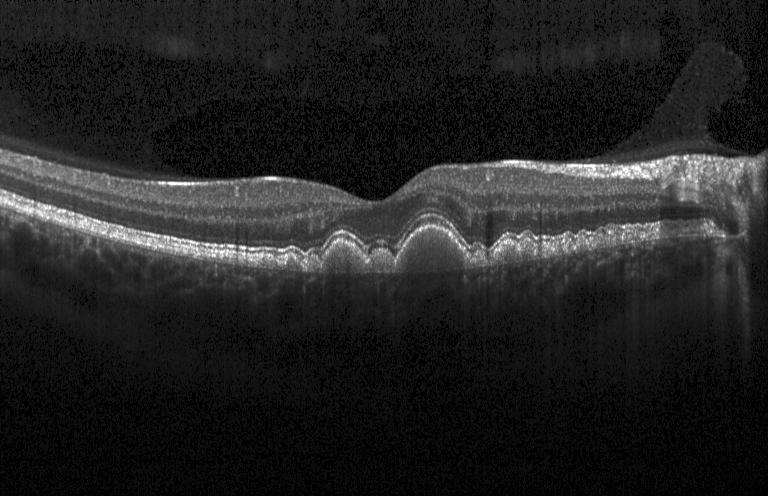
Spectral-domain OCT. Horizontal scan through the fovea. Retinal OCT cross-section. Heidelberg Spectralis OCT system
Diagnosis: drusen.